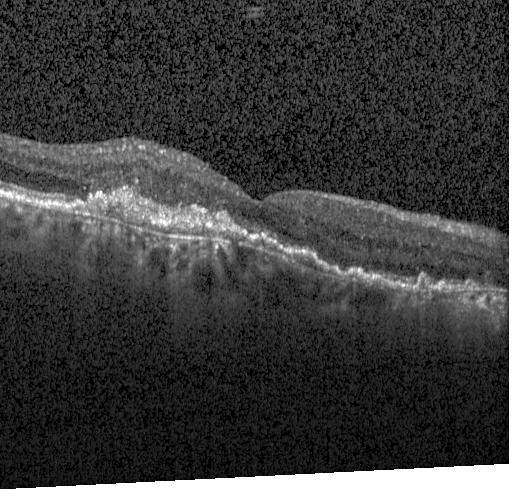 Spectral-domain OCT, fovea-centered, retinal OCT B-scan. Diagnosis: CNV.